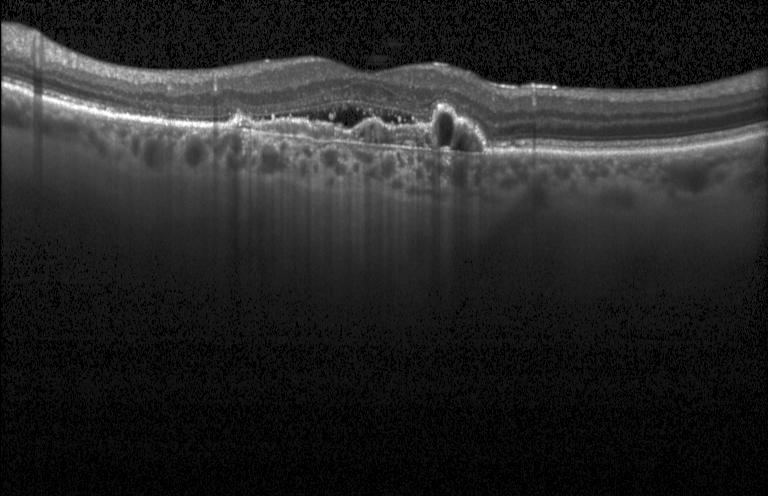
Macular OCT demonstrating CNV.